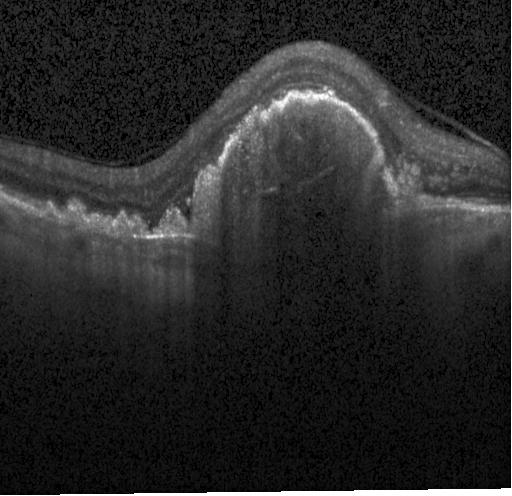
OCT line scan, SD-OCT — Impression: a choroidal neovascular membrane.